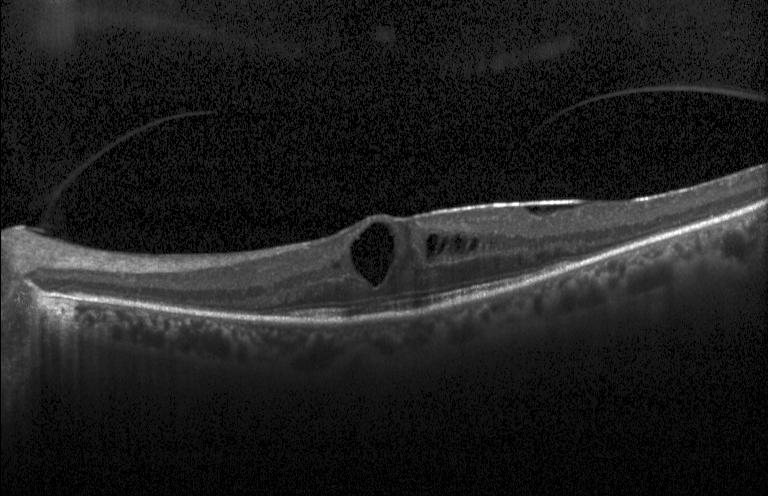 Retinal OCT B-scan, centered on the fovea. Finding: diabetic macular edema (DME).